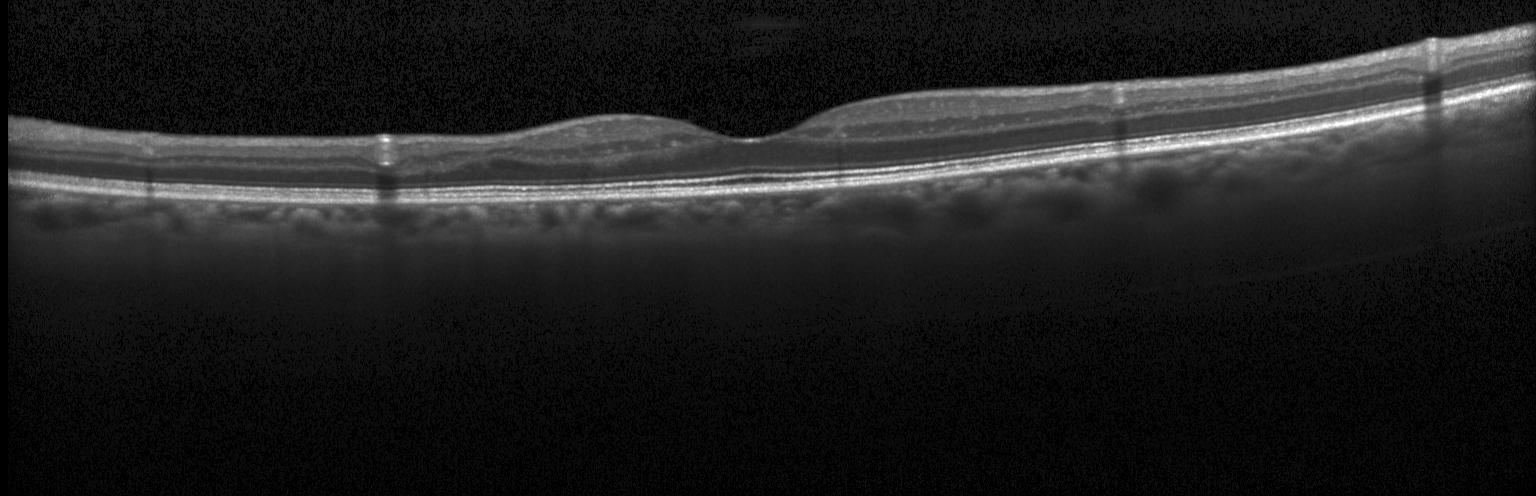

Retinal OCT cross-section · horizontal scan through the fovea · spectral-domain OCT · Heidelberg Spectralis OCT system.
This B-scan demonstrates neither choroidal neovascularization, diabetic macular edema, nor drusen.